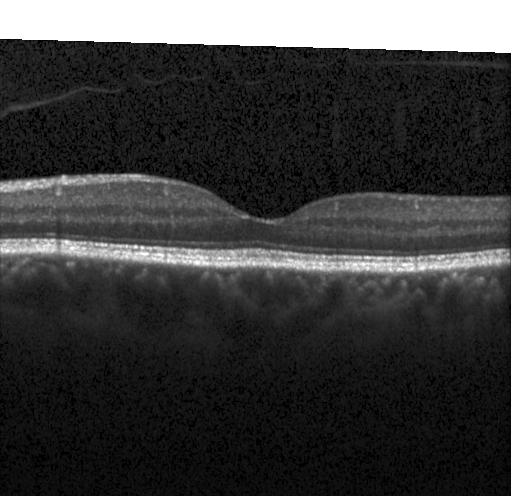

Spectral-domain OCT. Optical coherence tomography scan — Impression: no choroidal neovascularization, no diabetic macular edema, and no drusen.